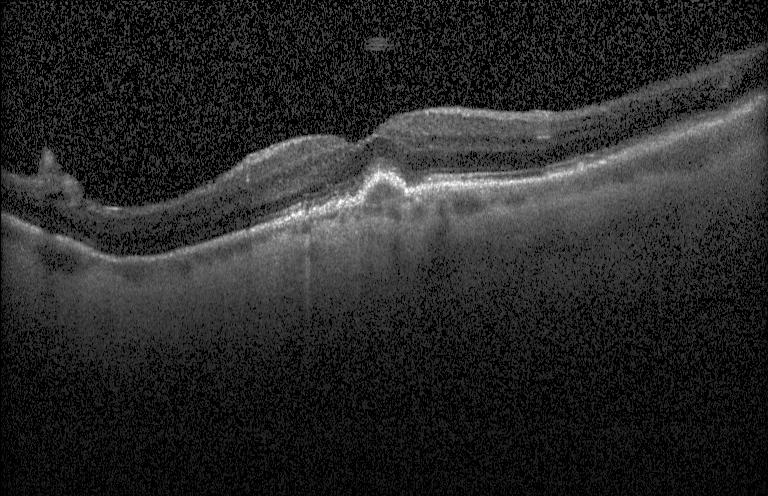

Macular OCT: drusen.